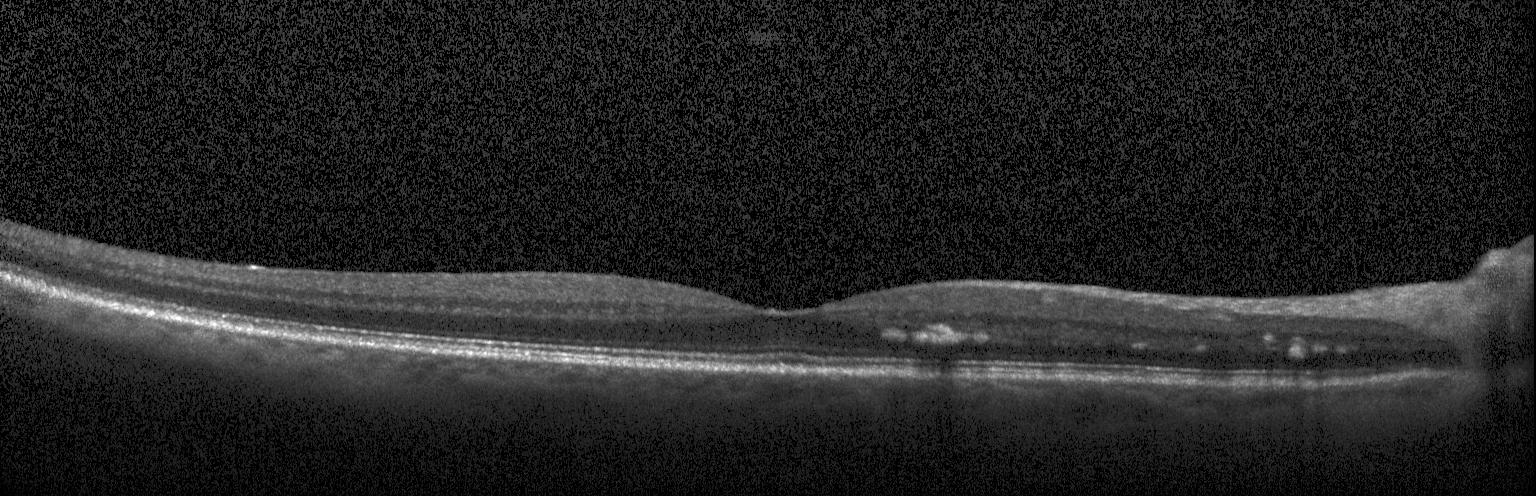

Dx: no CNV, no DME, and no drusen.